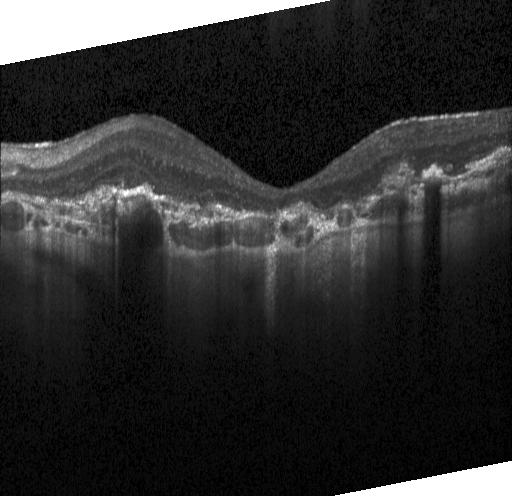 Optical coherence tomography scan, Heidelberg Spectralis, SD-OCT
Finding: choroidal neovascularization.